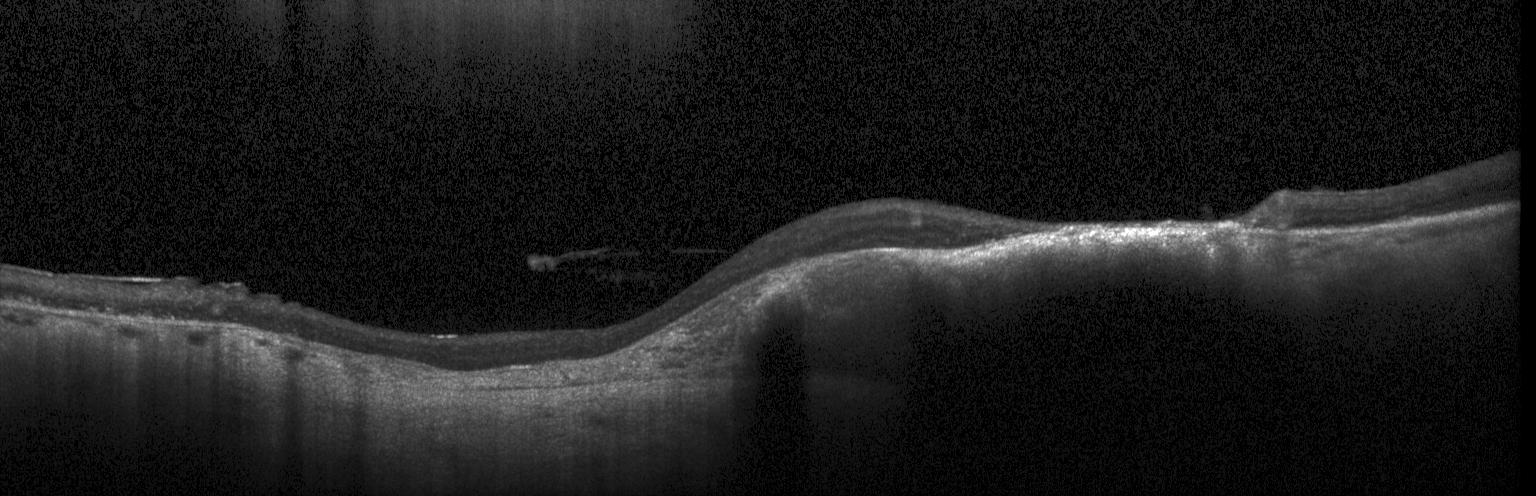 Heidelberg Spectralis, OCT line scan.
Macular OCT: a choroidal neovascular membrane.